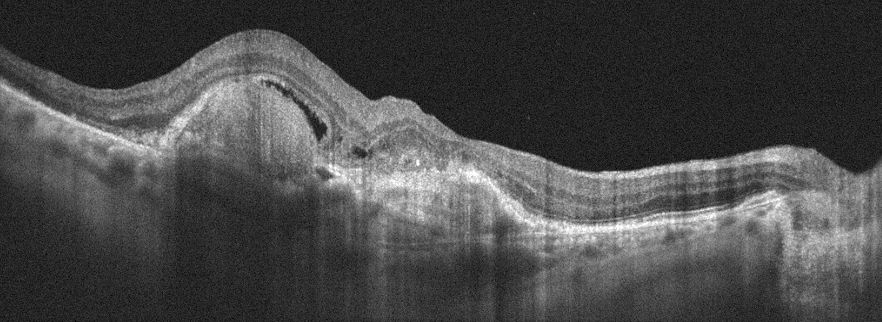
Acquired on an Optovue Avanti RTVue XR · OCT line scan · OS. Macular OCT: AMD.